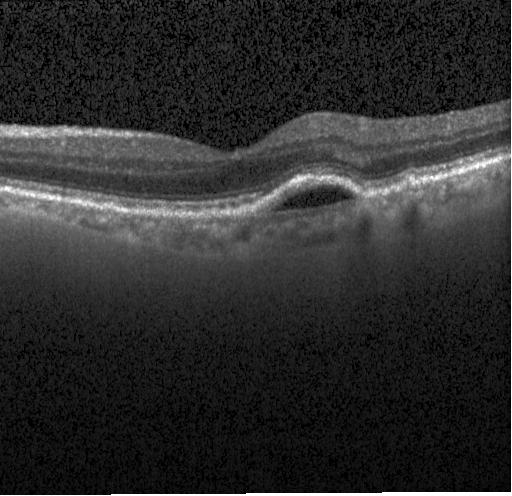 Spectral-domain OCT, OCT B-scan, macular scan, Heidelberg Spectralis OCT system. Diagnosis: a choroidal neovascular membrane.